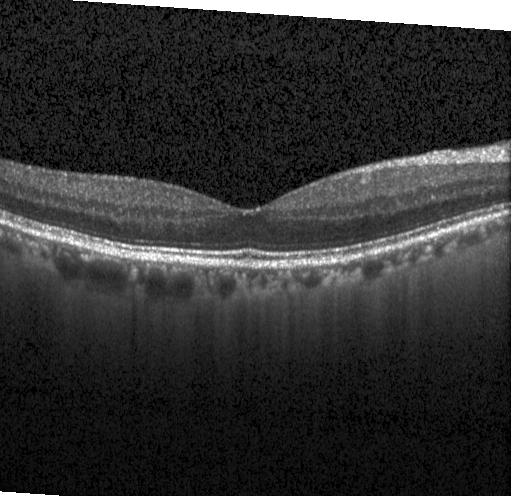

Heidelberg Spectralis, spectral-domain OCT, fovea-centered, OCT line scan.
This B-scan demonstrates no choroidal neovascularization, no diabetic macular edema, and no drusen.